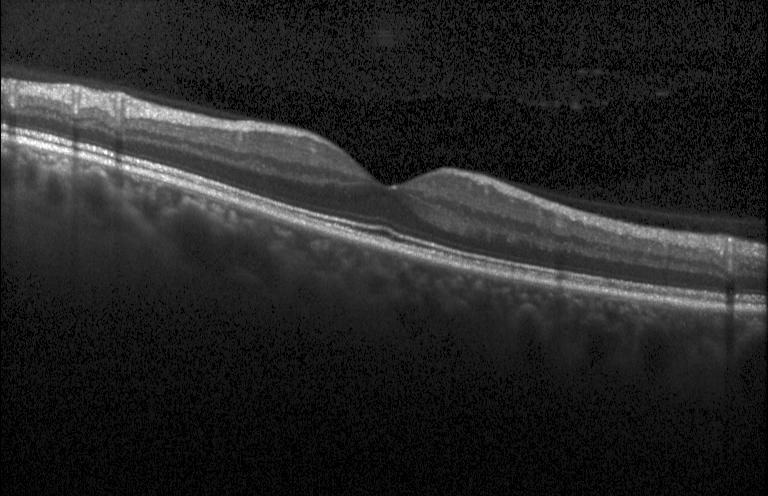
Optical coherence tomography B-scan. Finding: no CNV, DME, or drusen.